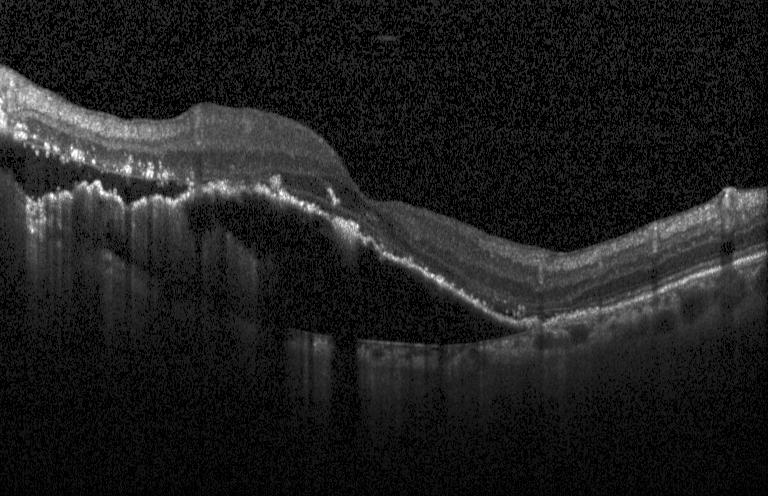
Heidelberg Spectralis OCT system; SD-OCT; through the macula; retinal OCT B-scan — This B-scan demonstrates choroidal neovascularization (CNV).